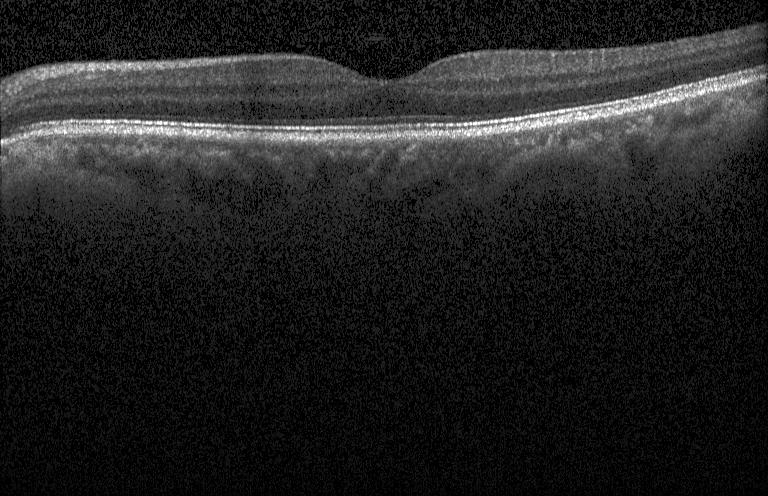 Through the macula; SD-OCT; optical coherence tomography B-scan; Heidelberg Spectralis — Diagnosis: no CNV, DME, or drusen.